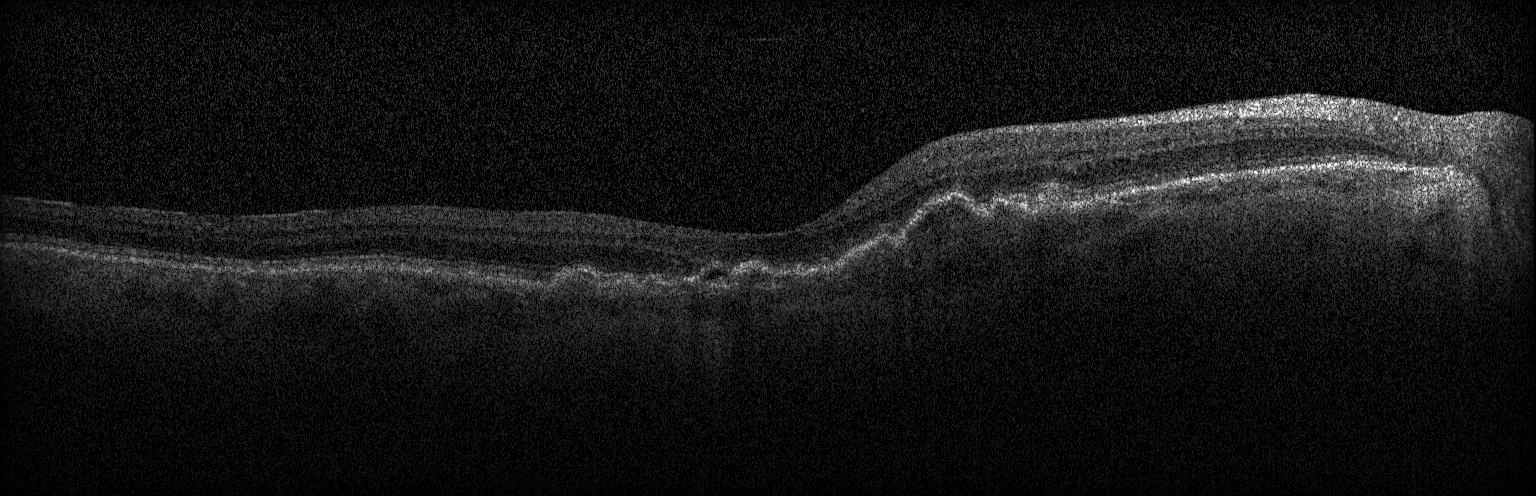 SD-OCT; fovea-centered; OCT line scan; Heidelberg Spectralis
Finding: a choroidal neovascular membrane.